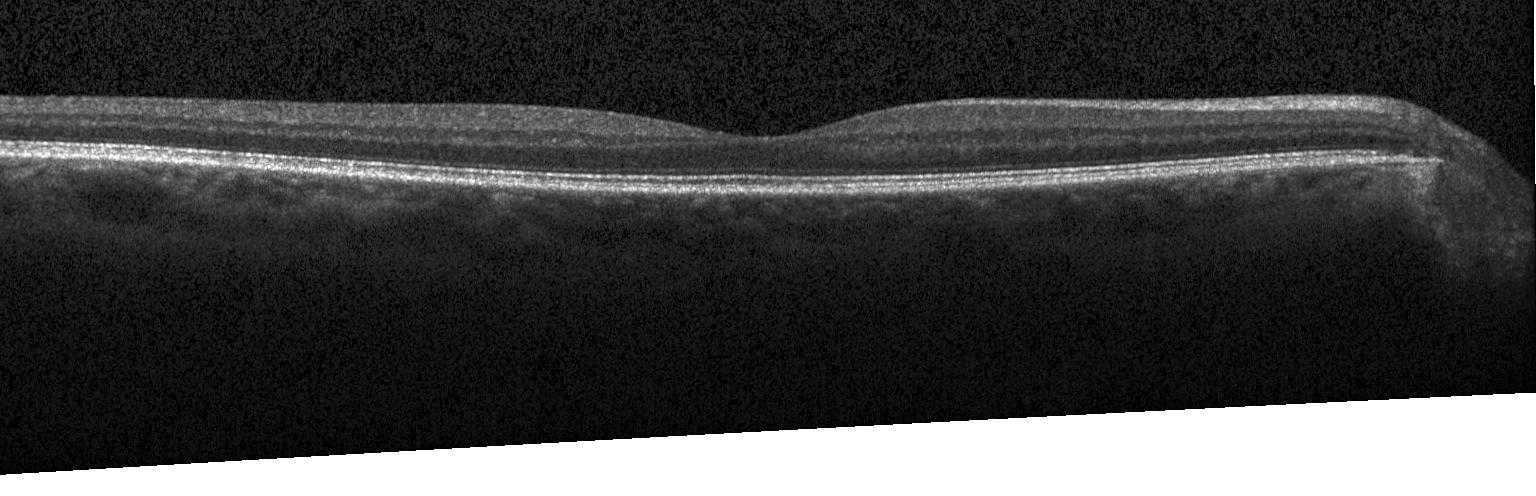

Fovea-centered · retinal OCT B-scan · spectral-domain optical coherence tomography · Heidelberg Spectralis — Macular OCT: no CNV, no DME, and no drusen.